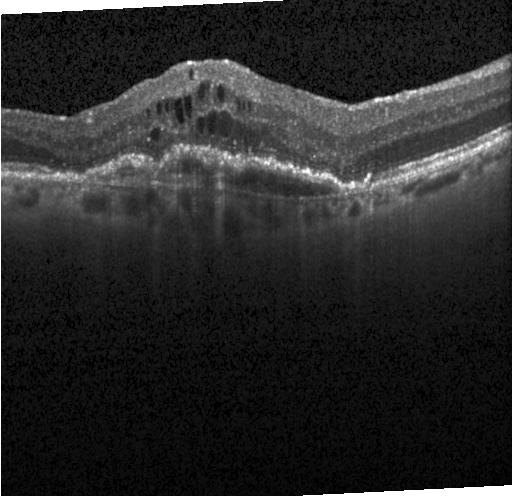

Macular OCT demonstrating a choroidal neovascular membrane.